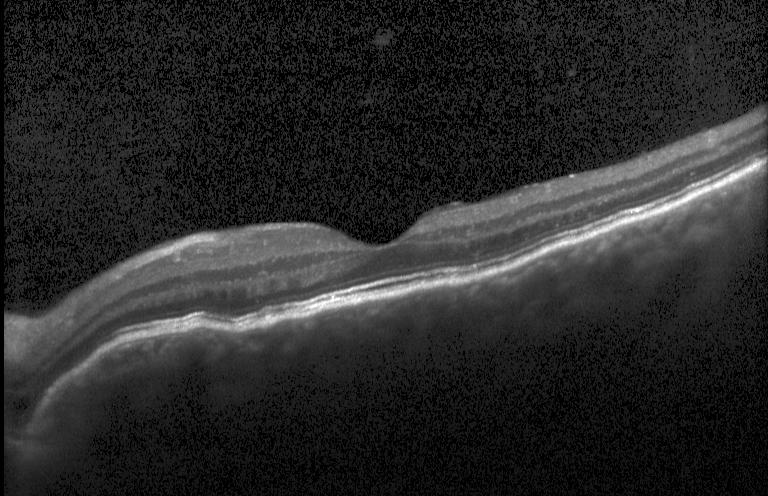

Heidelberg Spectralis, OCT line scan, horizontal scan through the fovea, spectral-domain OCT
No evidence of choroidal neovascularization, diabetic macular edema, or drusen.